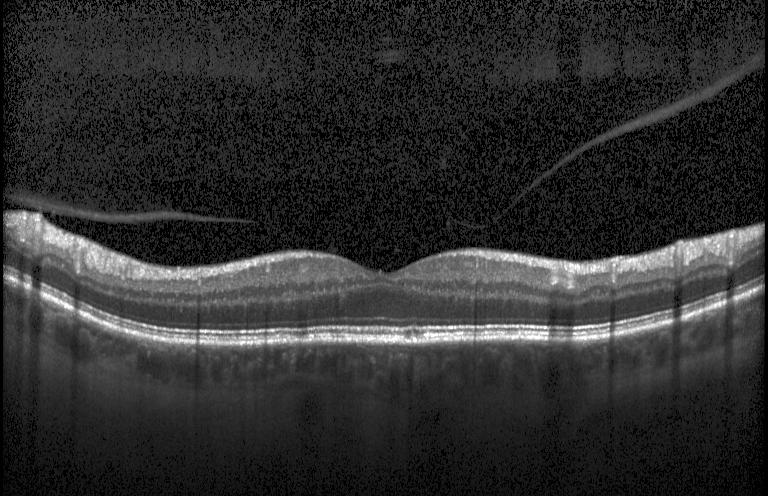

Retinal OCT cross-section showing no choroidal neovascularization, diabetic macular edema, or drusen.